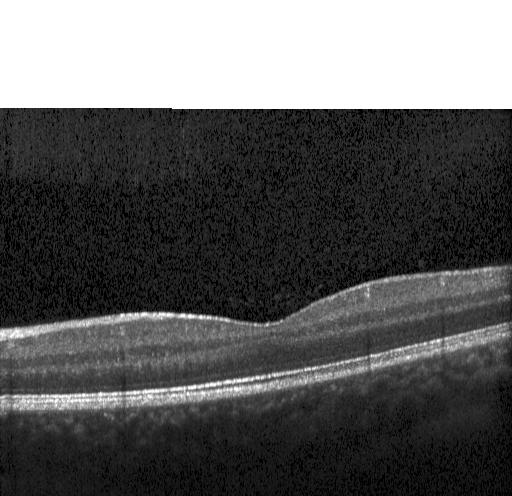
Horizontal scan through the fovea, retinal OCT cross-section
This B-scan demonstrates no CNV, no DME, and no drusen.